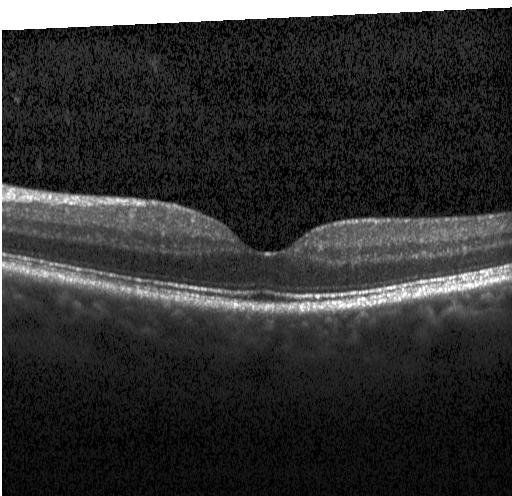

OCT finding: neither CNV, DME, nor drusen.